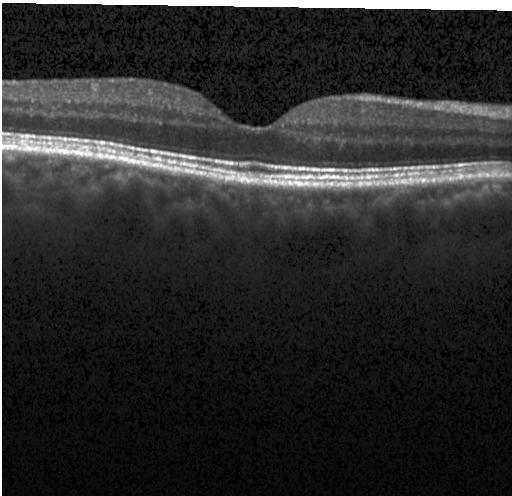

Spectral-domain optical coherence tomography. Through the macula. Retinal OCT B-scan. Finding: no choroidal neovascularization, no diabetic macular edema, and no drusen.